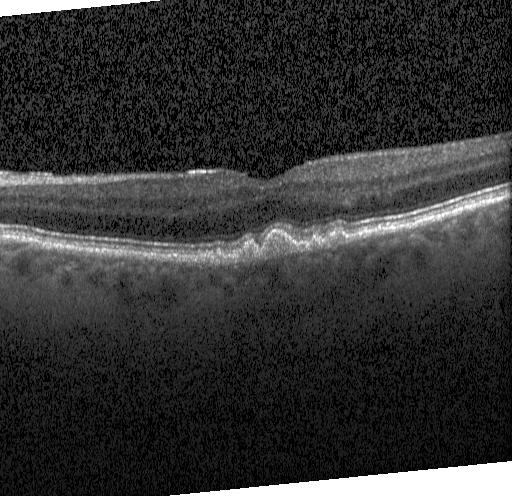
OCT line scan.
Diagnosis: multiple drusen.